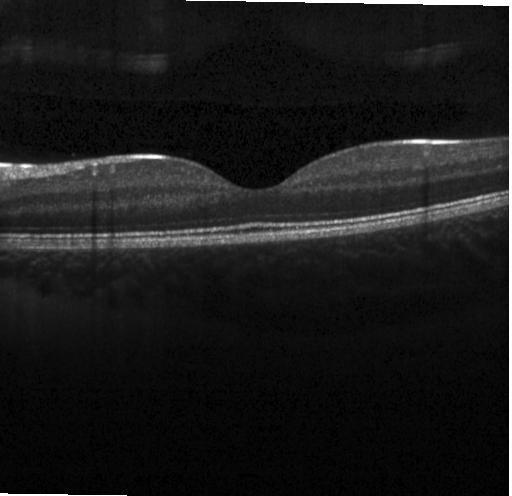

Impression: no evidence of choroidal neovascularization, diabetic macular edema, or drusen.